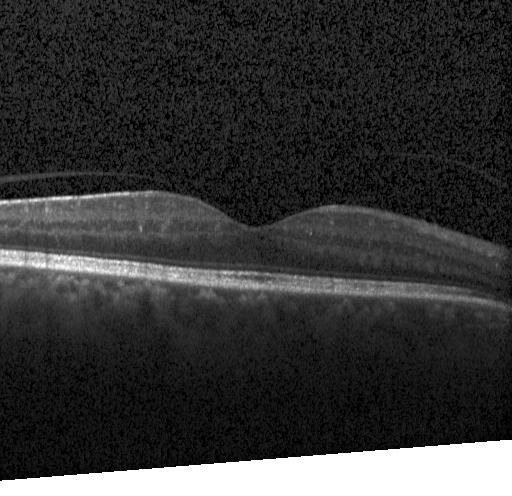 The scan shows no choroidal neovascularization, diabetic macular edema, or drusen.